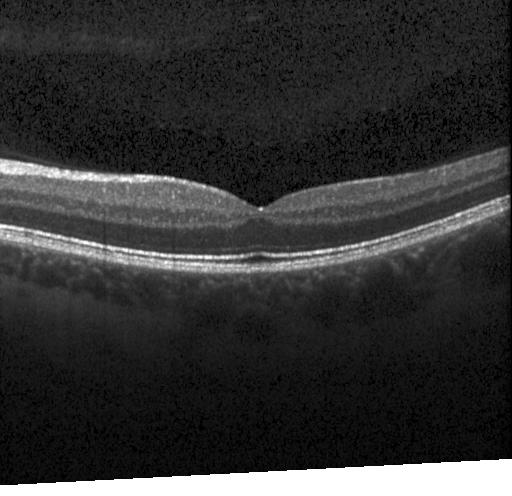
Spectral-domain OCT, centered on the fovea, retinal OCT cross-section, acquired on a Heidelberg Spectralis. Dx: no choroidal neovascularization, diabetic macular edema, or drusen.